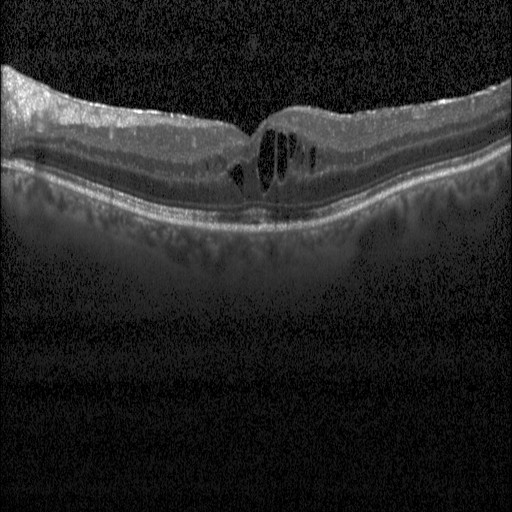
OCT line scan, through the macula — Finding: diabetic macular edema (DME).